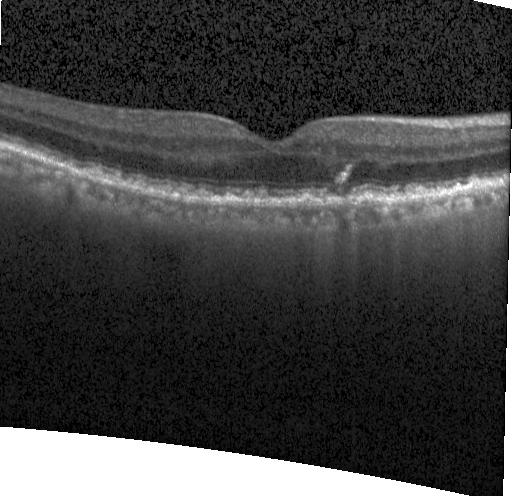 OCT B-scan, horizontal scan through the fovea.
Macular OCT: sub-RPE drusenoid deposits.